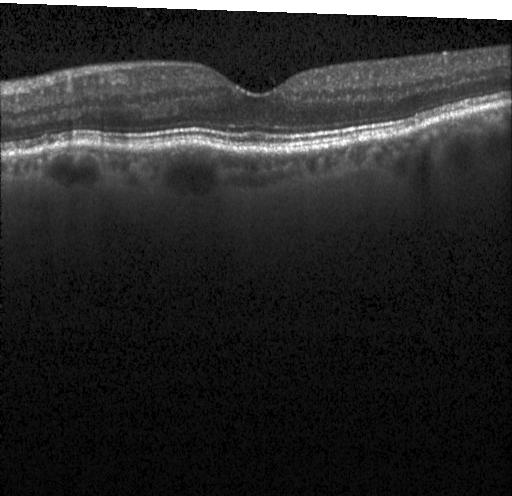 OCT scan showing neither choroidal neovascularization, diabetic macular edema, nor drusen.